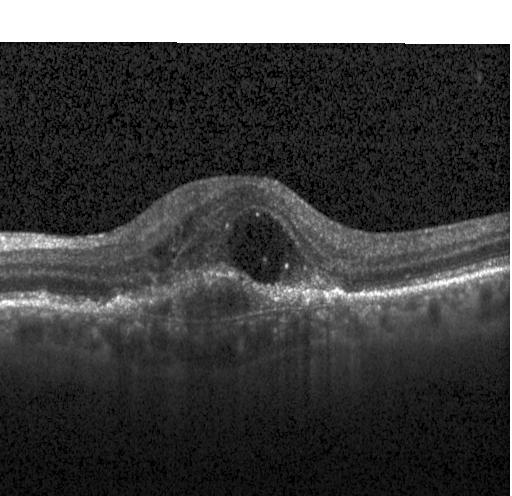

Fovea-centered. Retinal OCT B-scan
The scan shows a choroidal neovascular membrane.